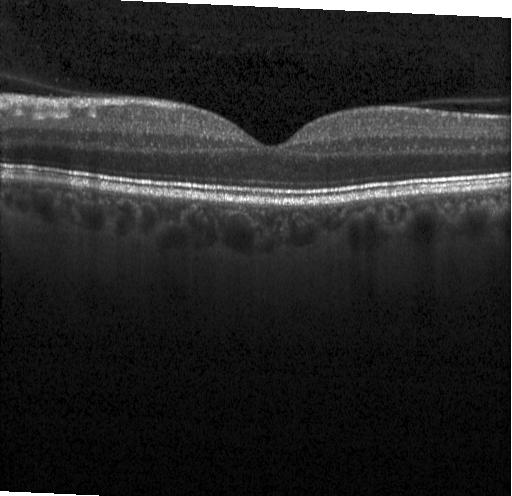

Retinal OCT cross-section. Heidelberg Spectralis OCT system
OCT finding: no evidence of choroidal neovascularization, diabetic macular edema, or drusen.